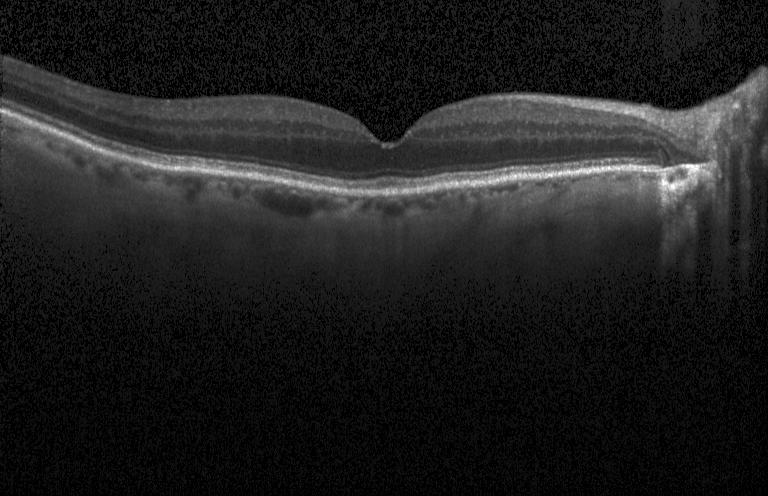
Through the macula, retinal OCT cross-section, Heidelberg Spectralis, SD-OCT
Finding: no evidence of CNV, DME, or drusen.